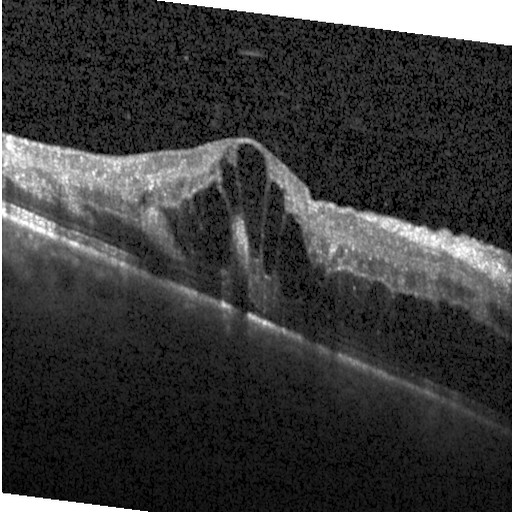

Retinal OCT B-scan · acquired on a Heidelberg Spectralis · centered on the fovea.
Diagnosis: diabetic macular edema.